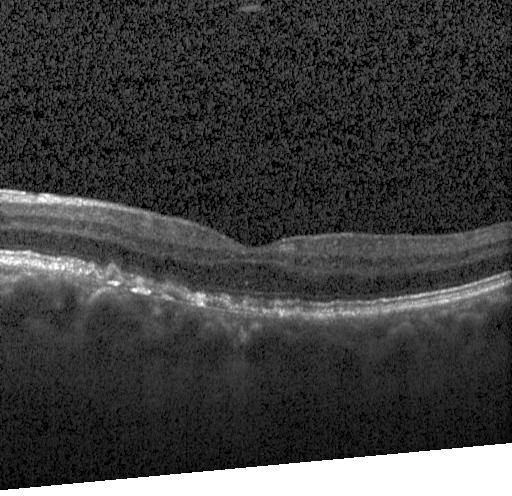
OCT line scan
OCT finding: CNV.